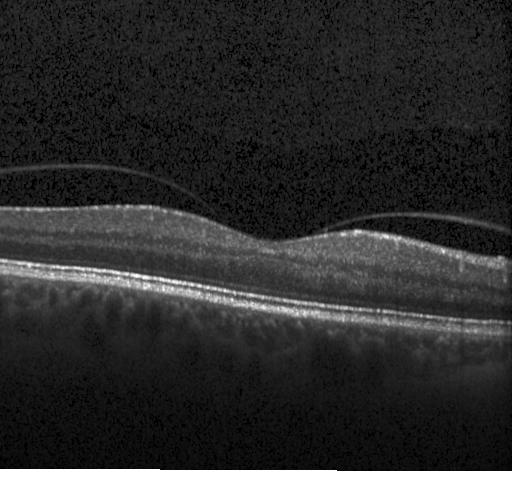
Retinal OCT cross-section. Impression: no choroidal neovascularization, no diabetic macular edema, and no drusen.